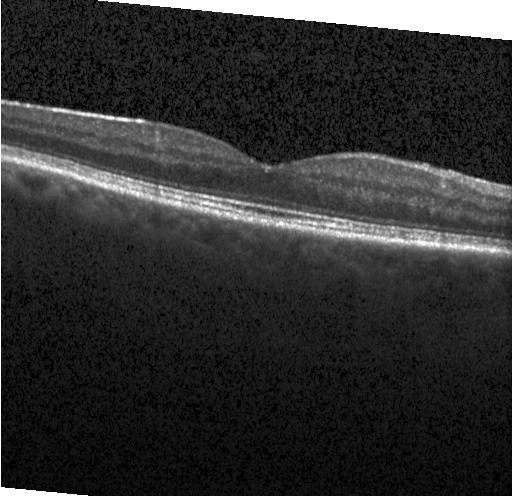 OCT B-scan; spectral-domain OCT. Dx: no choroidal neovascularization, diabetic macular edema, or drusen.